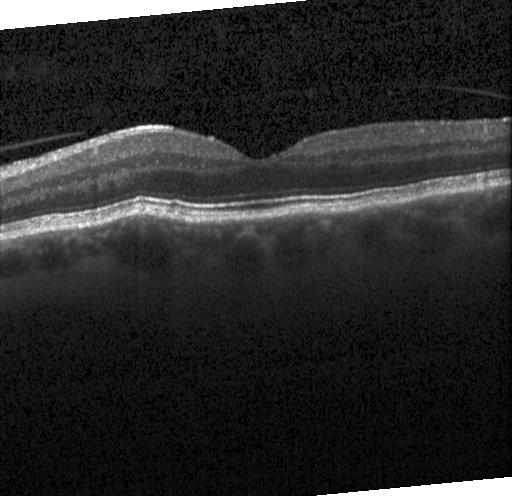
OCT line scan — Macular OCT: no evidence of choroidal neovascularization, diabetic macular edema, or drusen.